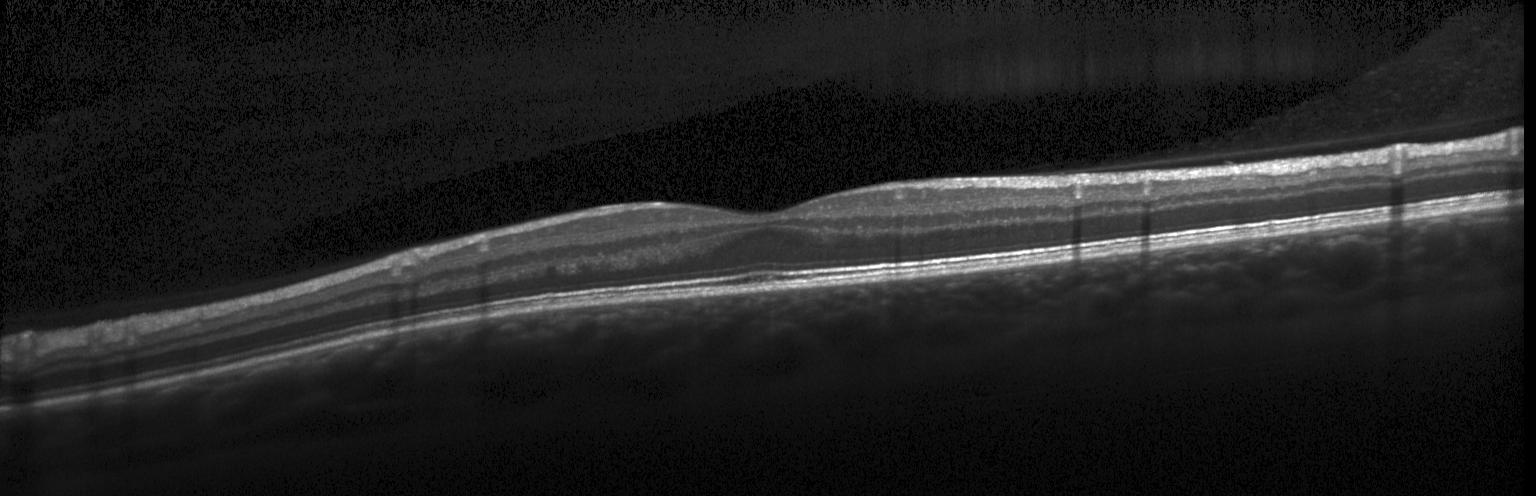 Optical coherence tomography scan. Assessment: no choroidal neovascularization, diabetic macular edema, or drusen.